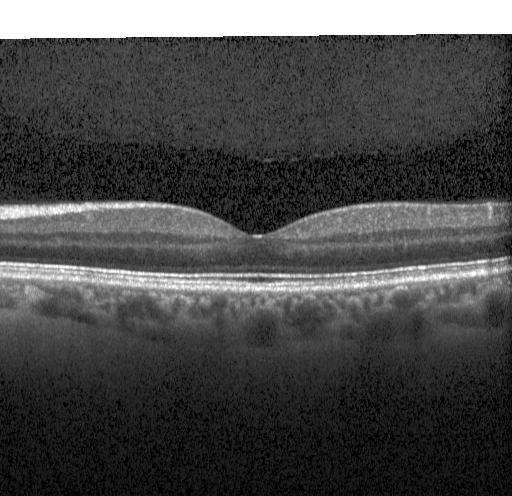

Optical coherence tomography scan · fovea-centered · Heidelberg Spectralis · spectral-domain OCT. OCT finding: no choroidal neovascularization, diabetic macular edema, or drusen.